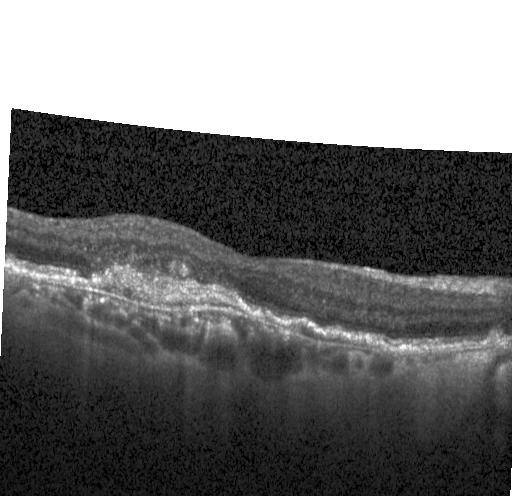 SD-OCT. Macular scan. Optical coherence tomography B-scan — The scan shows CNV.